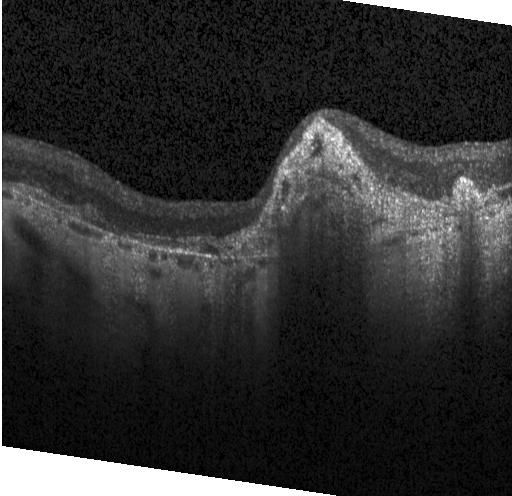 OCT B-scan showing CNV.